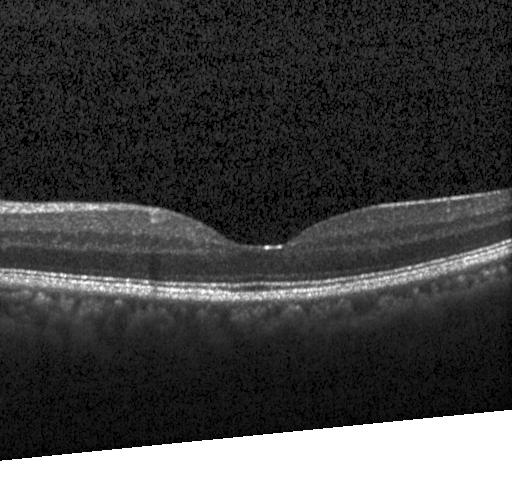
Instrument: Heidelberg Spectralis; fovea-centered; OCT B-scan.
Diagnosis: no evidence of choroidal neovascularization, diabetic macular edema, or drusen.